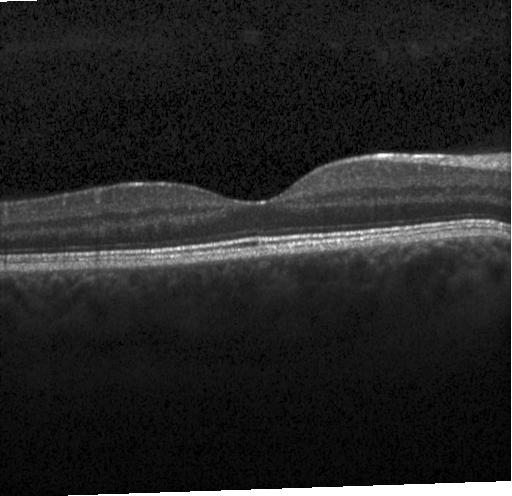 Optical coherence tomography B-scan. The scan shows no choroidal neovascularization, diabetic macular edema, or drusen.